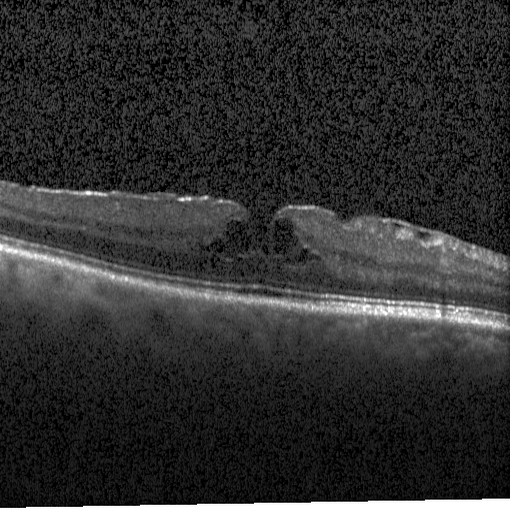
Optical coherence tomography scan · acquired on a Heidelberg Spectralis · centered on the fovea · SD-OCT
Macular OCT: diabetic macular edema.